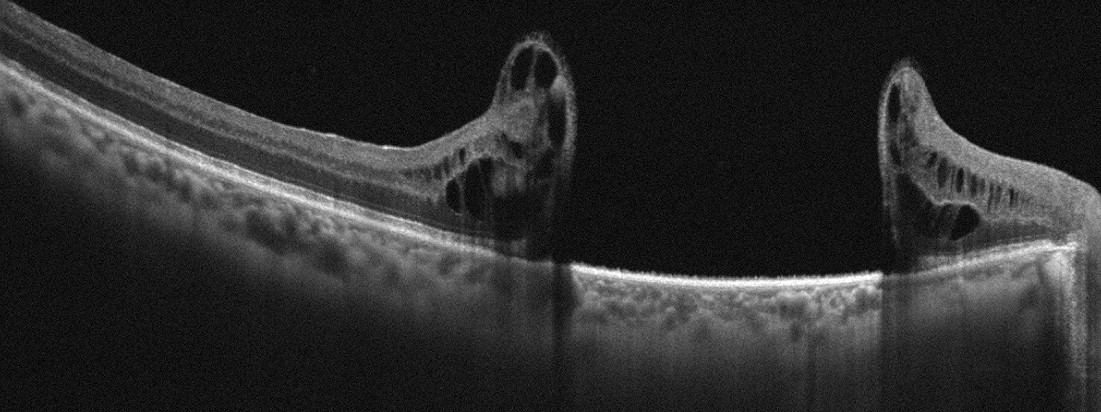 Spectral-domain OCT B-scan: VID.